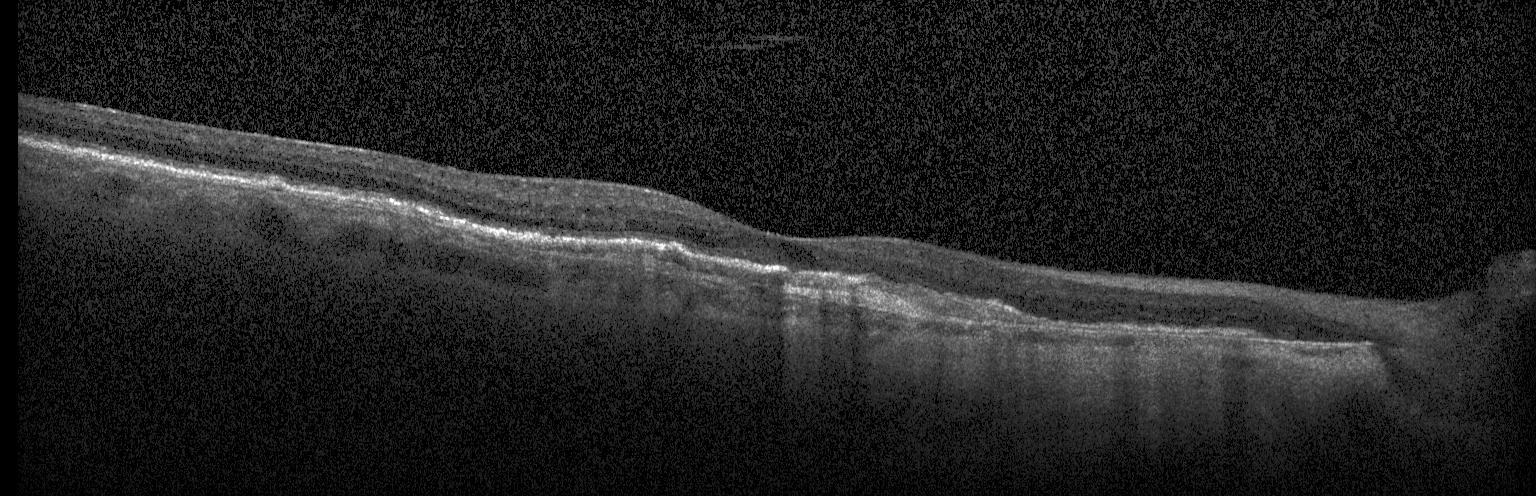 Centered on the fovea, retinal OCT cross-section — Impression: CNV.